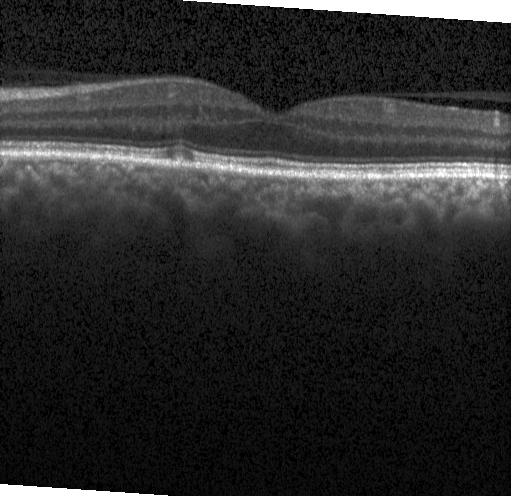 Spectral-domain OCT · OCT B-scan · instrument: Heidelberg Spectralis. Diagnosis: multiple drusen.